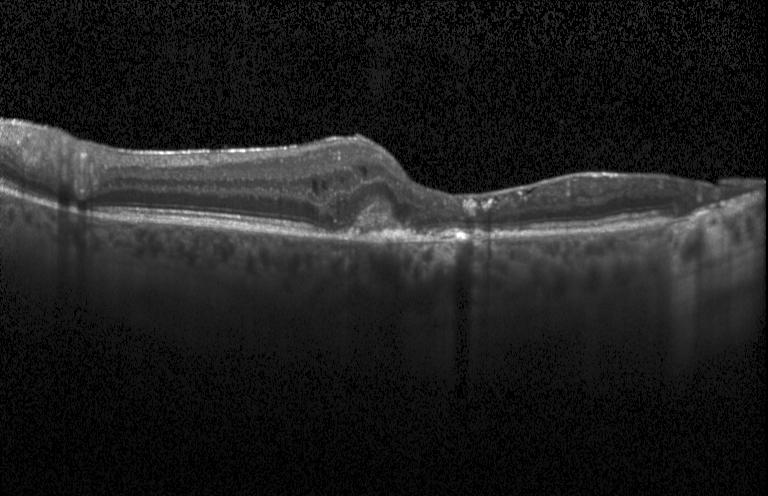

Optical coherence tomography B-scan. SD-OCT. Acquired on a Heidelberg Spectralis. Fovea-centered. This B-scan demonstrates CNV.